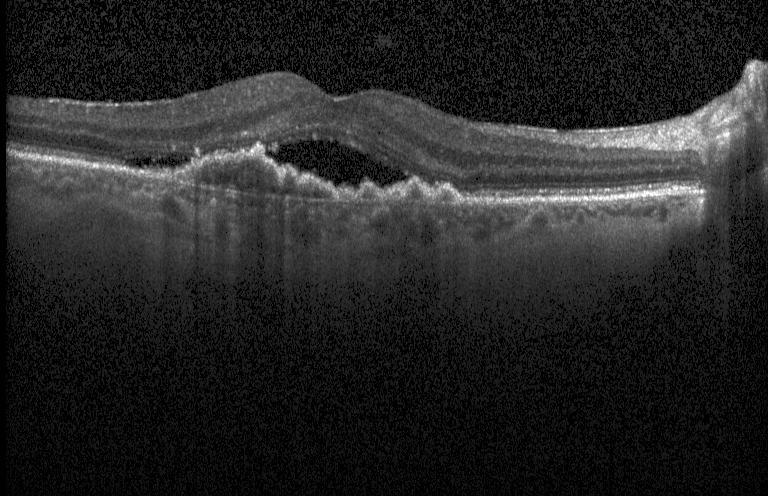

Assessment: choroidal neovascularization (CNV).